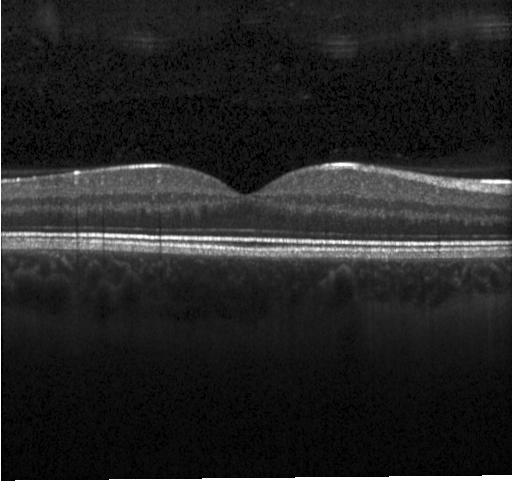
Diagnosis: no choroidal neovascularization, diabetic macular edema, or drusen.